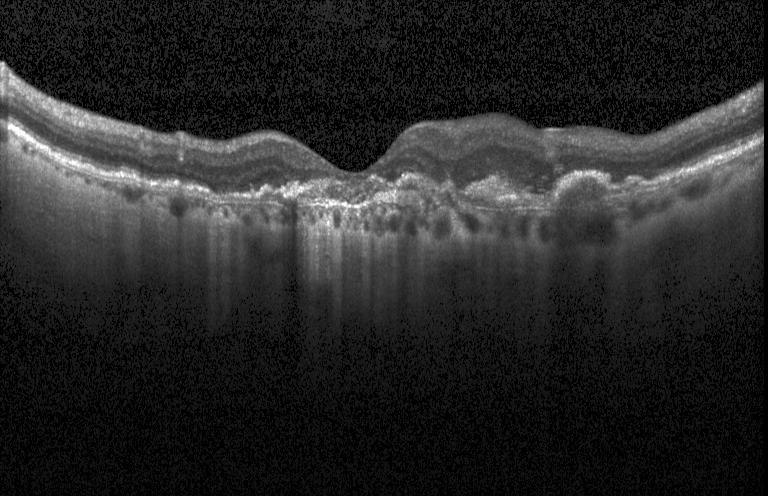

Diagnosis: choroidal neovascularization.